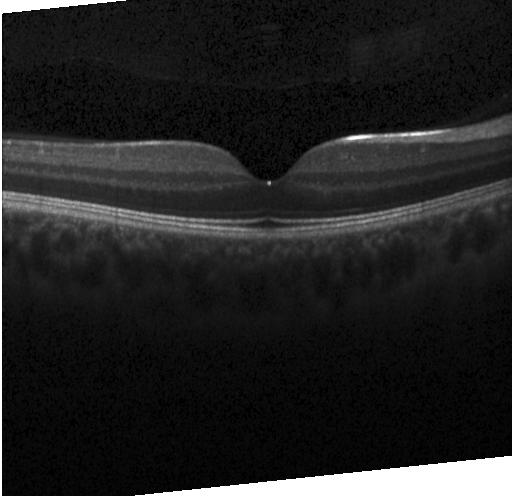 Retinal OCT B-scan. OCT finding: no choroidal neovascularization, diabetic macular edema, or drusen.